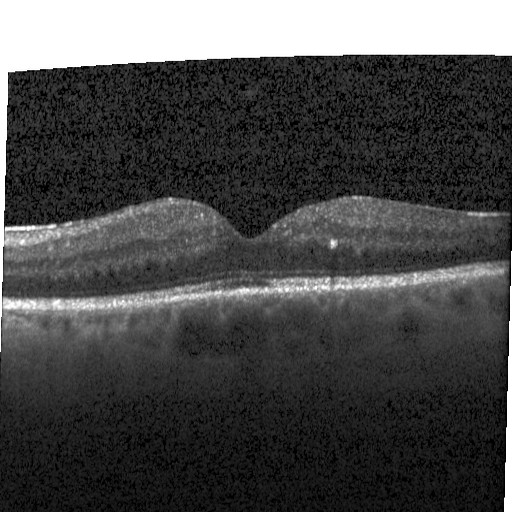

Optical coherence tomography scan.
OCT finding: diabetic macular edema.